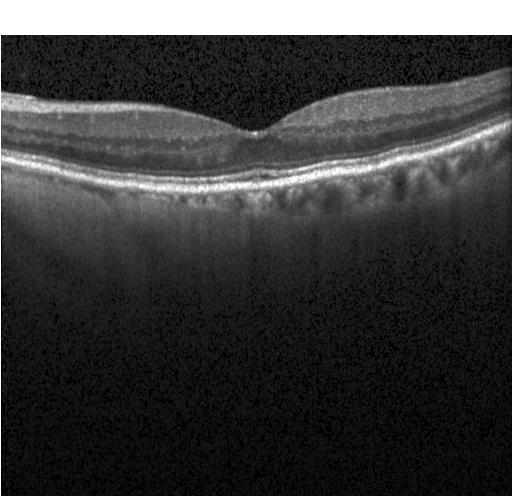
OCT B-scan, SD-OCT, acquired on a Heidelberg Spectralis, fovea-centered — Diagnosis: no CNV, no DME, and no drusen.